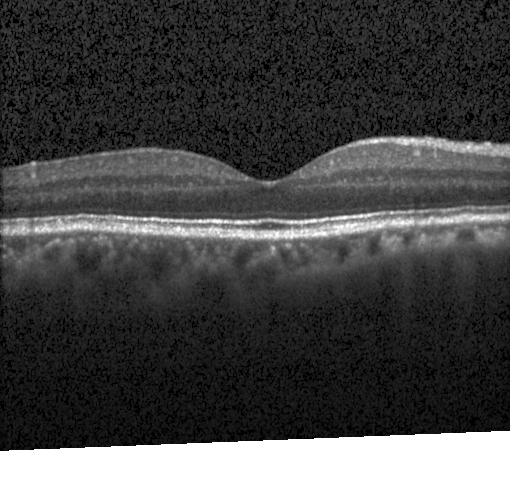

Dx: no evidence of CNV, DME, or drusen.